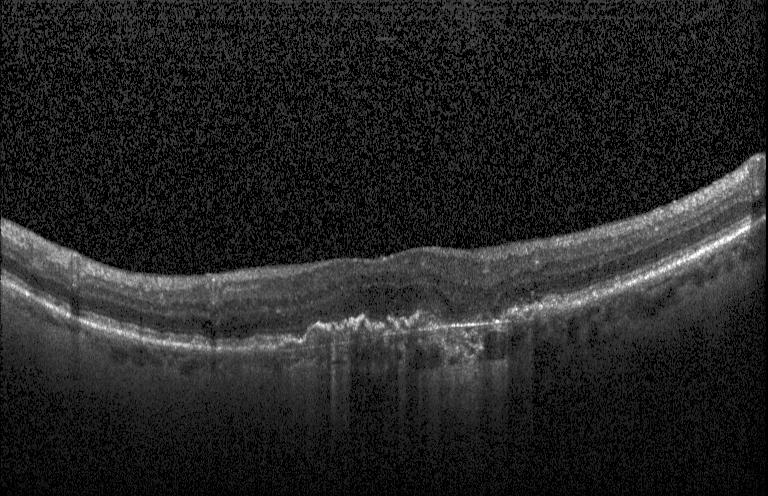 Spectral-domain optical coherence tomography, OCT line scan.
Assessment: choroidal neovascularization.